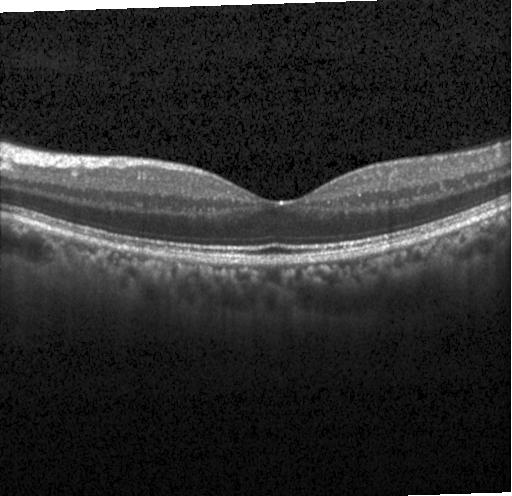 Optical coherence tomography scan. Macular scan
Neither choroidal neovascularization, diabetic macular edema, nor drusen.